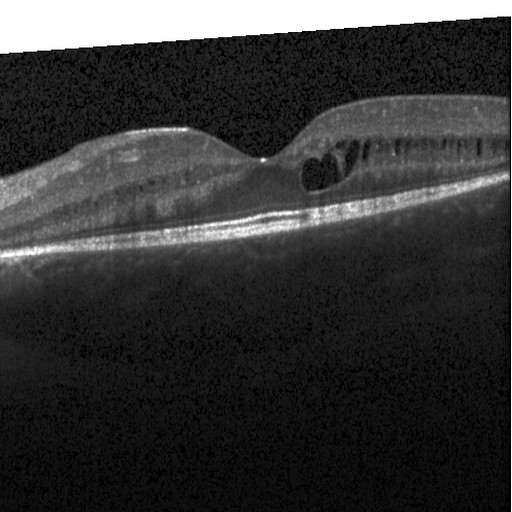
OCT B-scan showing diabetic macular edema.